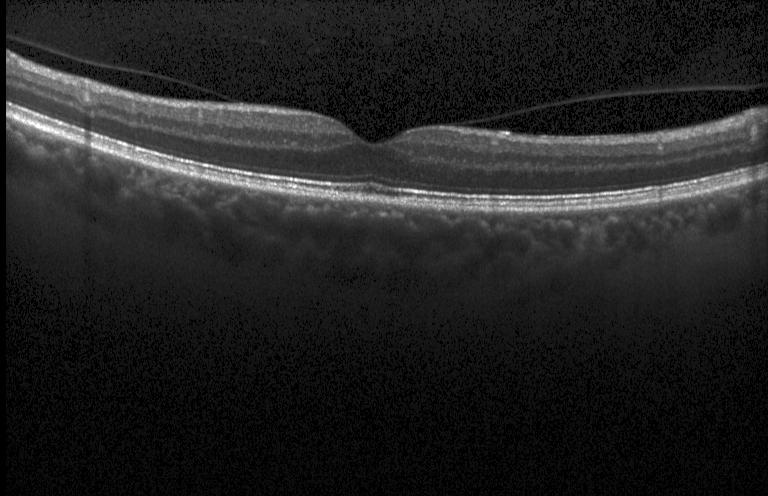 Neither choroidal neovascularization, diabetic macular edema, nor drusen.